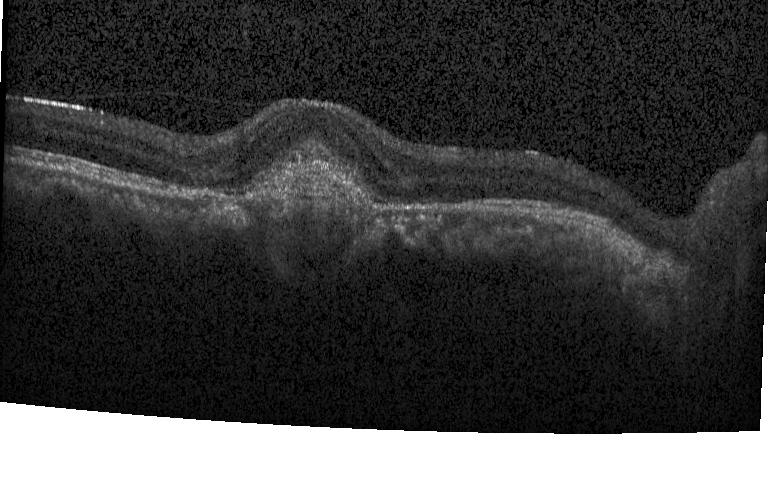

Heidelberg Spectralis; horizontal scan through the fovea; OCT B-scan — Assessment: choroidal neovascularization.